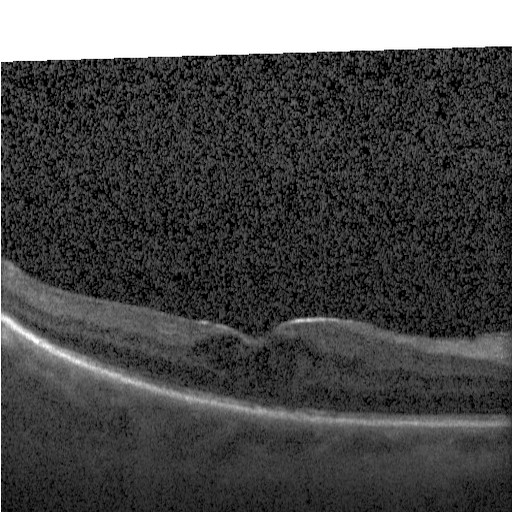
Acquired on a Heidelberg Spectralis, OCT line scan.
Macular OCT: diabetic macular edema.